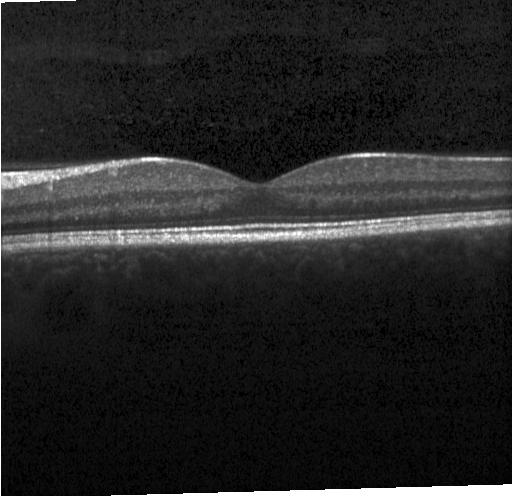 Diagnosis: no choroidal neovascularization, no diabetic macular edema, and no drusen.